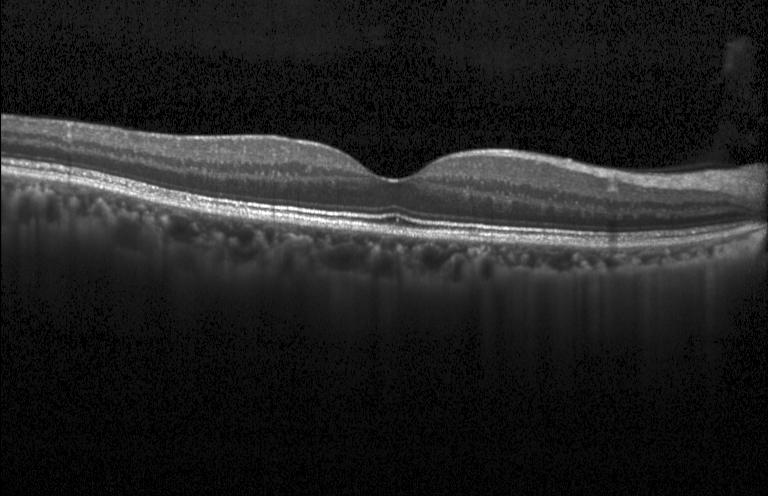

Optical coherence tomography scan; spectral-domain OCT; Heidelberg Spectralis.
Impression: no choroidal neovascularization, no diabetic macular edema, and no drusen.